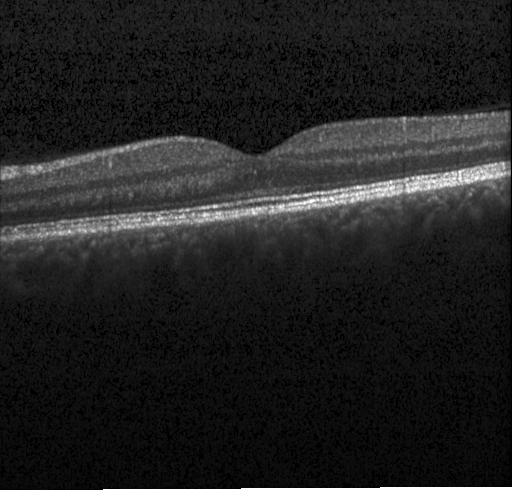 Macular OCT demonstrating no choroidal neovascularization, no diabetic macular edema, and no drusen.